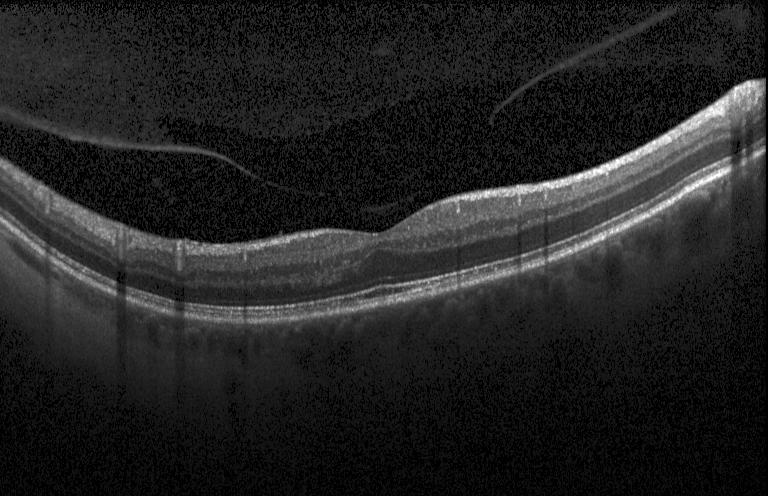 Macular OCT: neither CNV, DME, nor drusen.